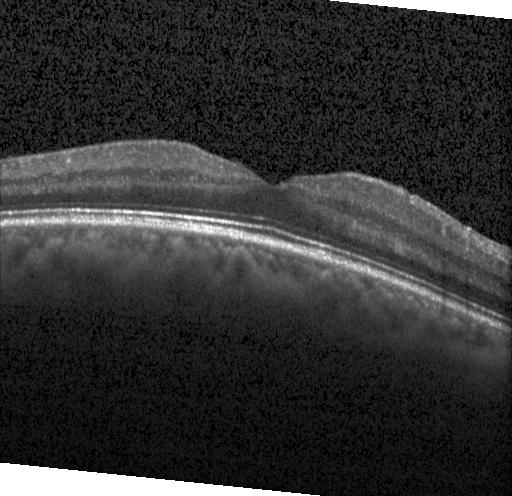 OCT B-scan, acquired on a Heidelberg Spectralis, spectral-domain OCT.
Finding: no CNV, no DME, and no drusen.